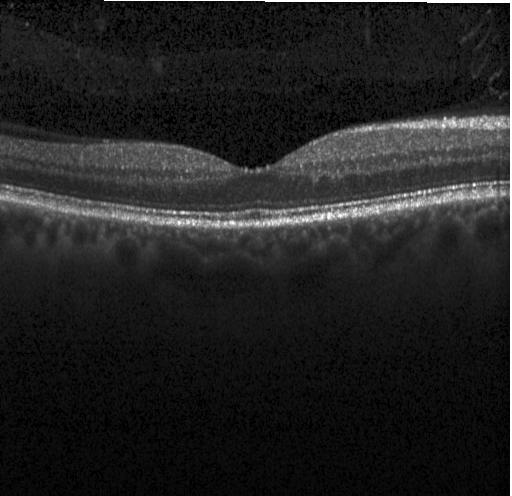 Finding: neither CNV, DME, nor drusen.